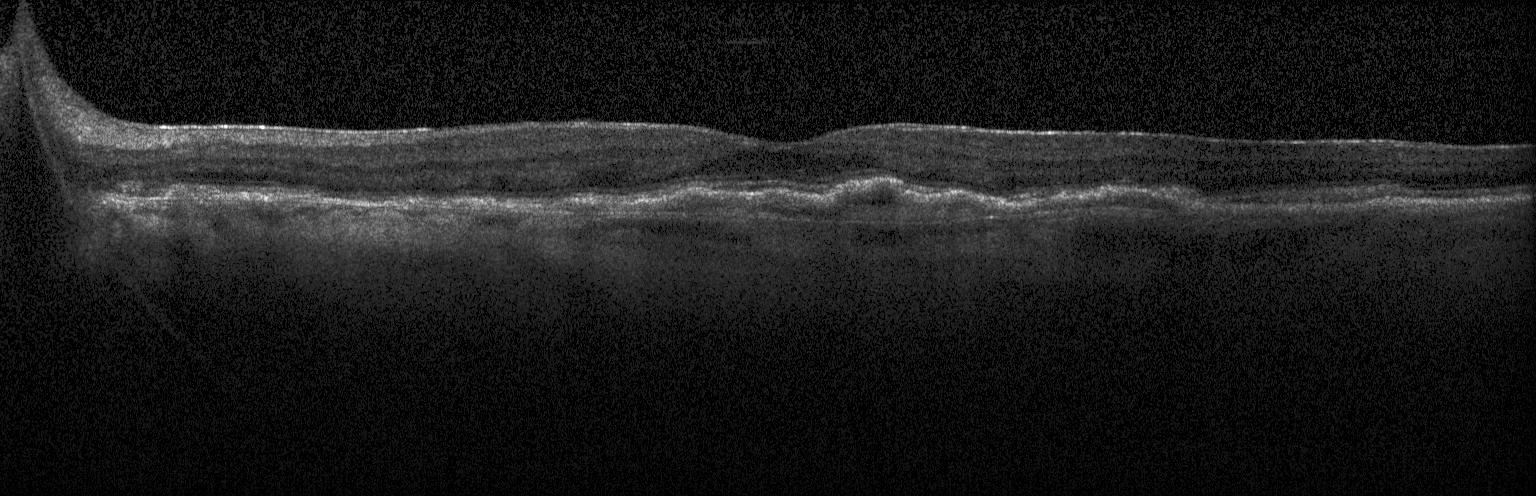
OCT finding: choroidal neovascularization (CNV).